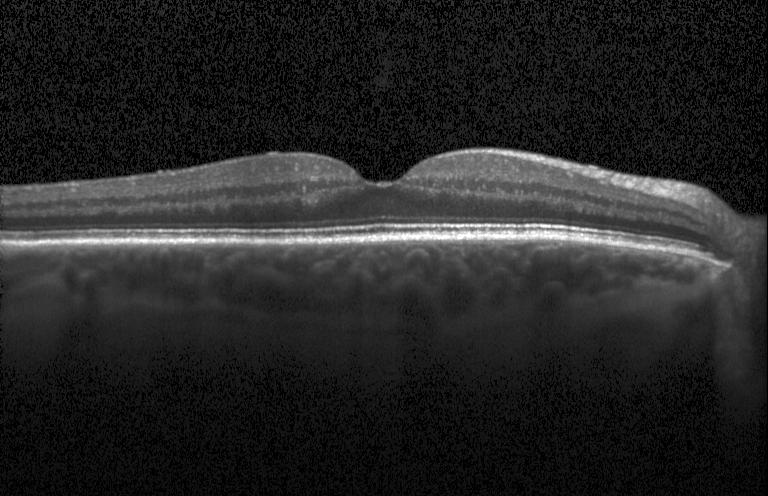 Fovea-centered. Optical coherence tomography scan. Heidelberg Spectralis — The scan shows no choroidal neovascularization, diabetic macular edema, or drusen.